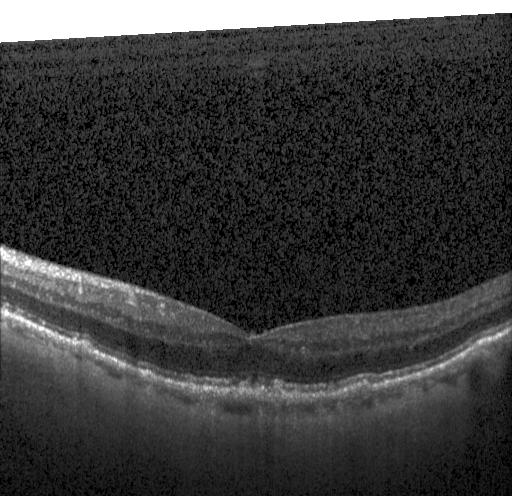
OCT scan showing sub-RPE drusenoid deposits.